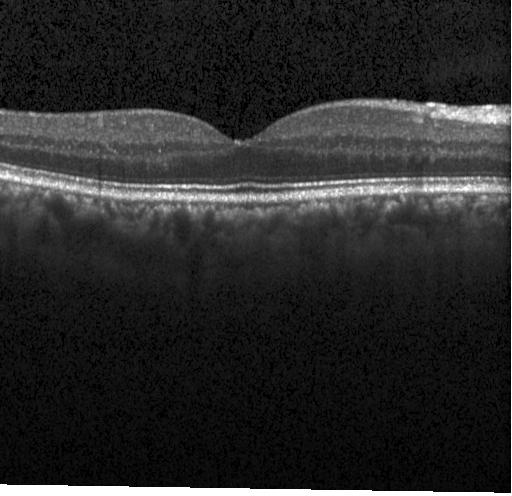
Through the macula, optical coherence tomography B-scan, instrument: Heidelberg Spectralis, spectral-domain OCT — Impression: no evidence of choroidal neovascularization, diabetic macular edema, or drusen.